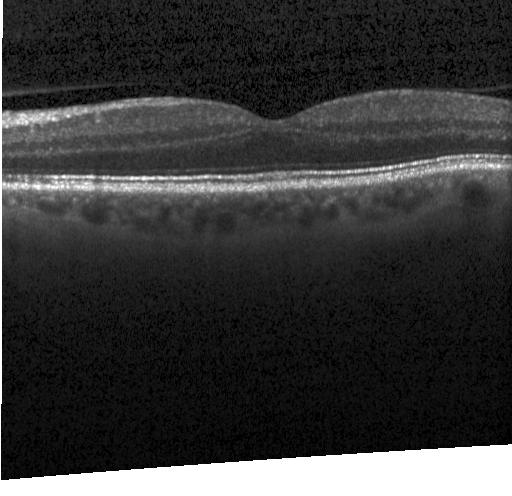 Spectral-domain OCT B-scan: neither choroidal neovascularization, diabetic macular edema, nor drusen.